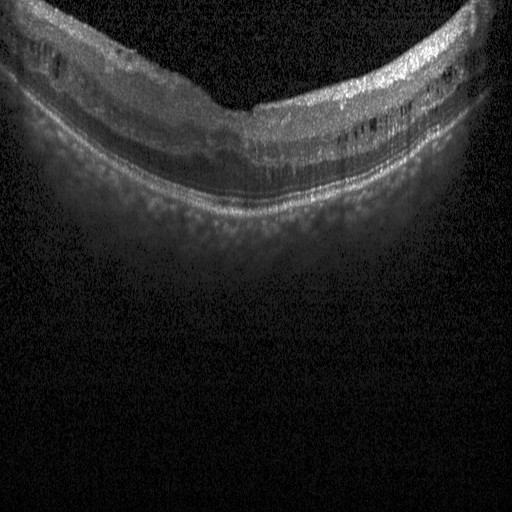

Macular OCT demonstrating diabetic macular edema.